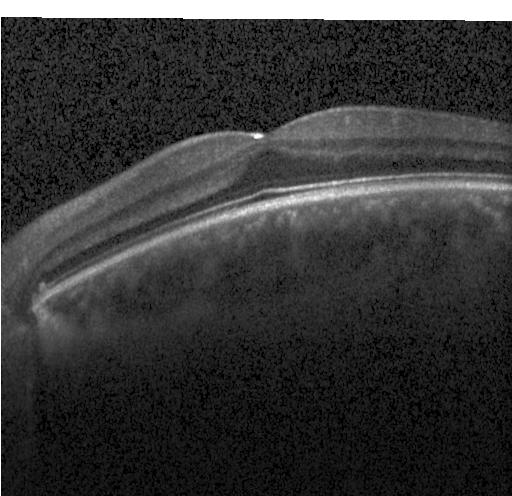 OCT B-scan showing no choroidal neovascularization, no diabetic macular edema, and no drusen.